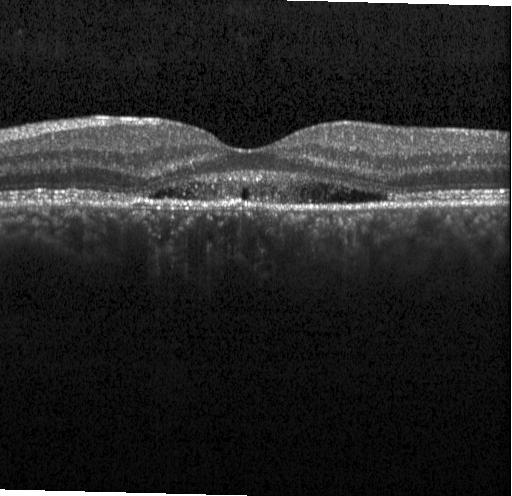
OCT B-scan showing a choroidal neovascular membrane.